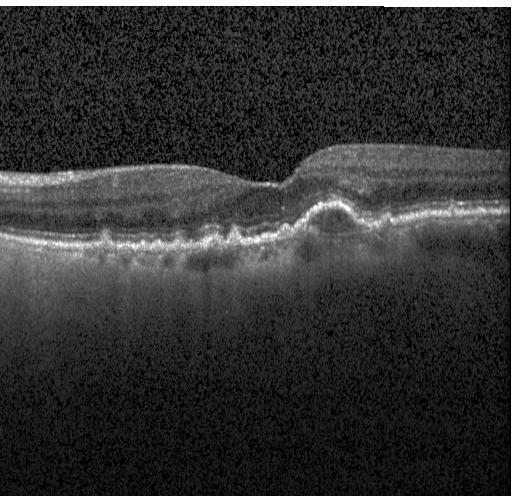
Retinal OCT cross-section. Fovea-centered — Diagnosis: choroidal neovascularization.